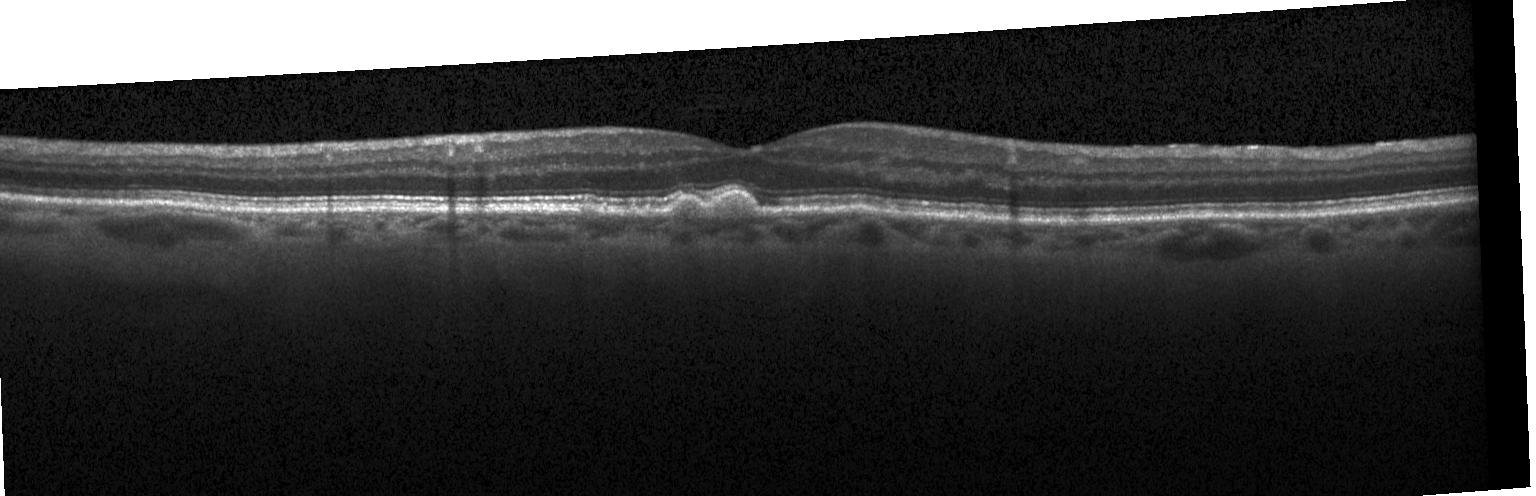
Spectral-domain OCT B-scan: multiple drusen.